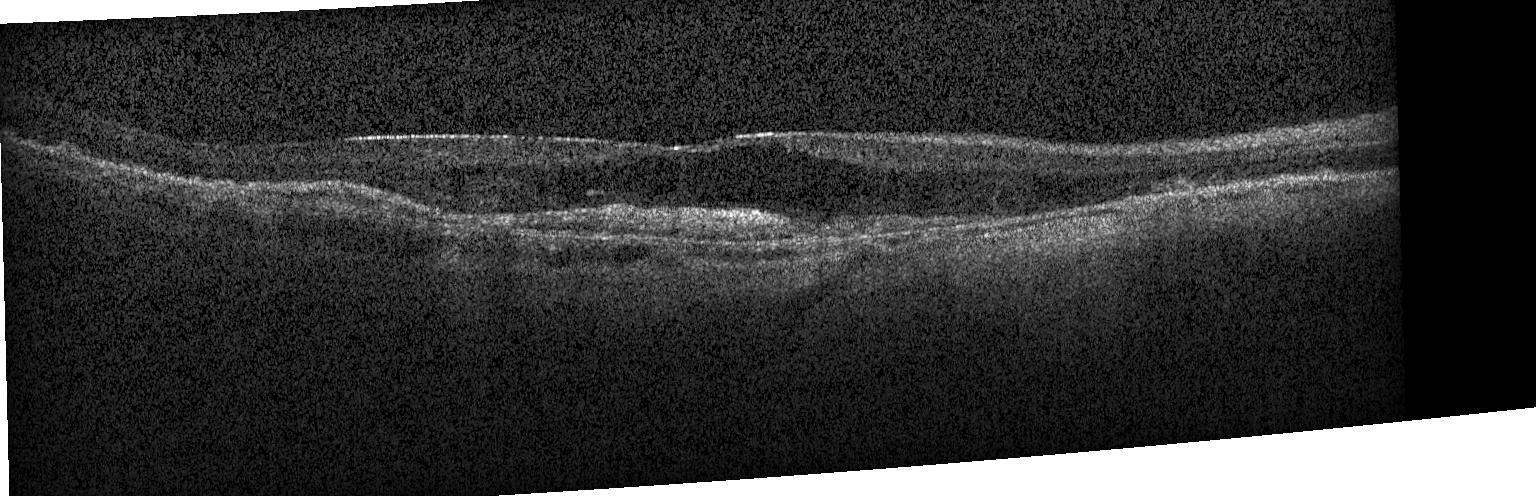 OCT line scan — Impression: choroidal neovascularization (CNV).